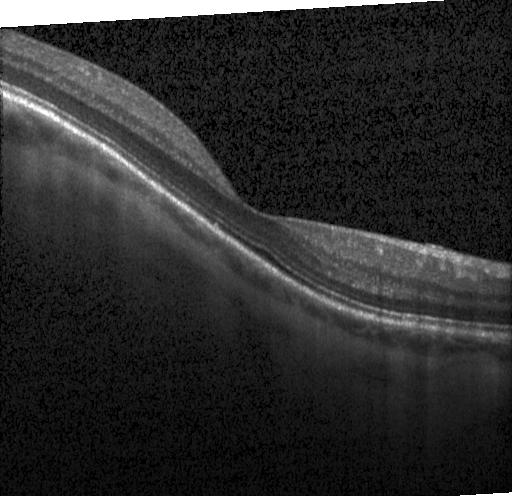

Retinal OCT B-scan. Finding: no choroidal neovascularization, no diabetic macular edema, and no drusen.